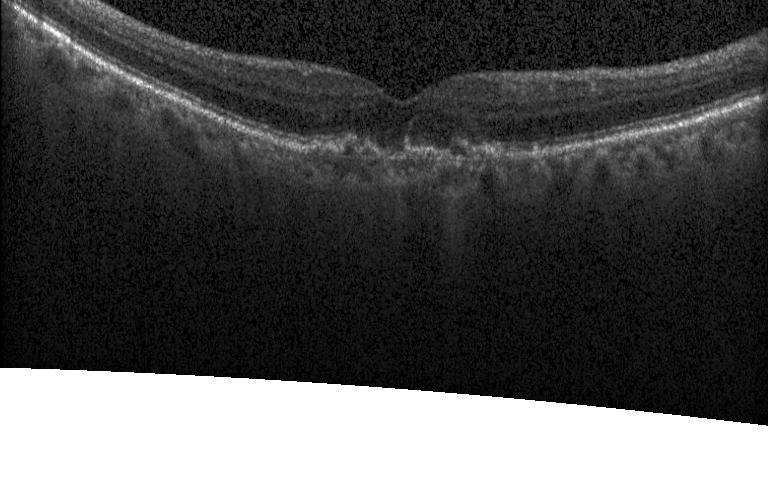

Macular scan, retinal OCT B-scan, spectral-domain optical coherence tomography
Macular OCT: a choroidal neovascular membrane.